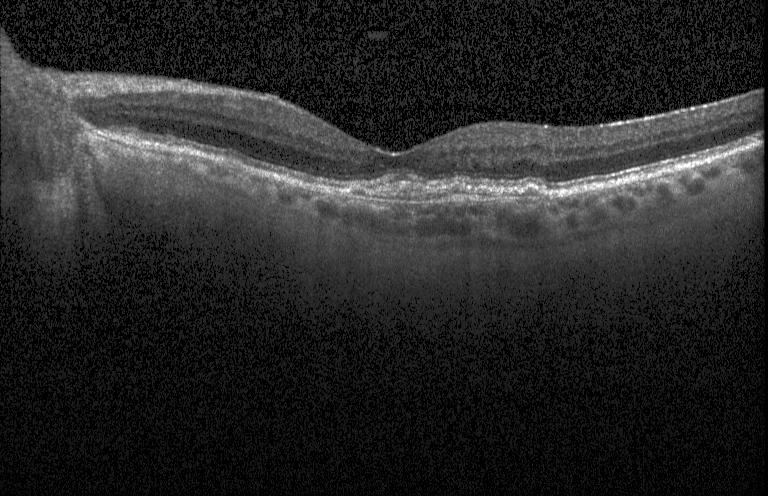

Diagnosis: a choroidal neovascular membrane.